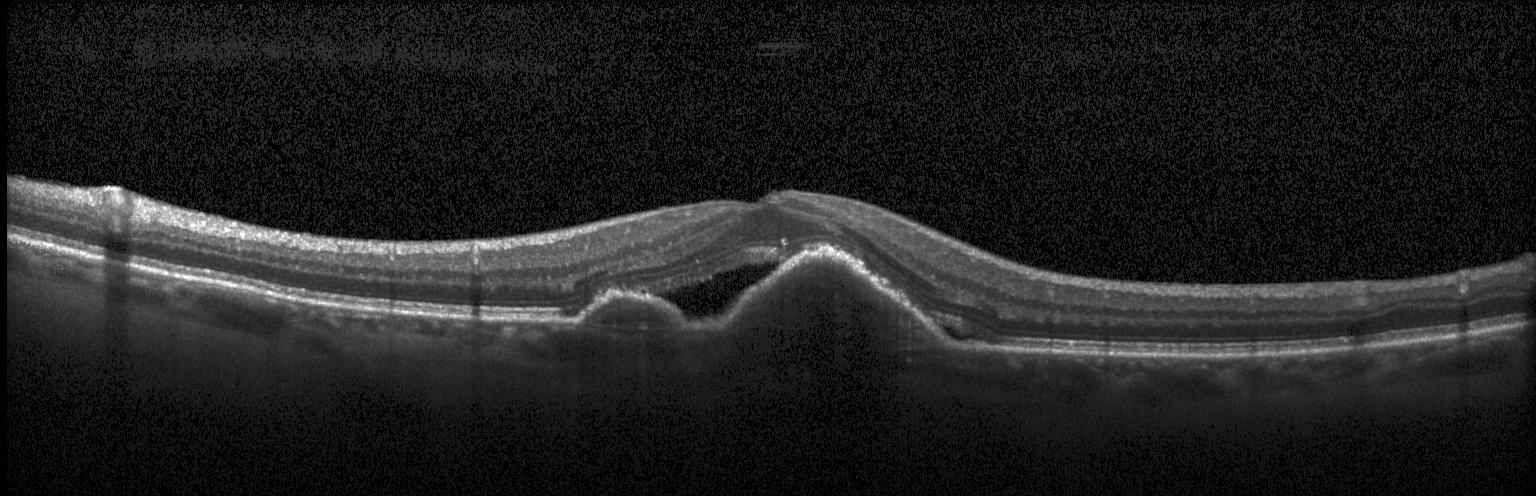

Assessment: a choroidal neovascular membrane.